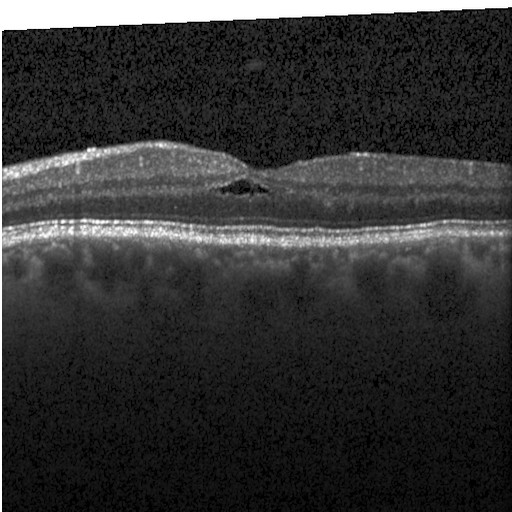

OCT B-scan.
Diagnosis: diabetic macular edema.